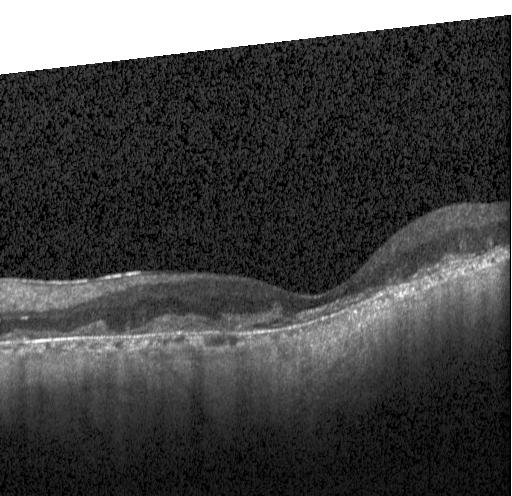 Optical coherence tomography scan
Impression: a choroidal neovascular membrane.